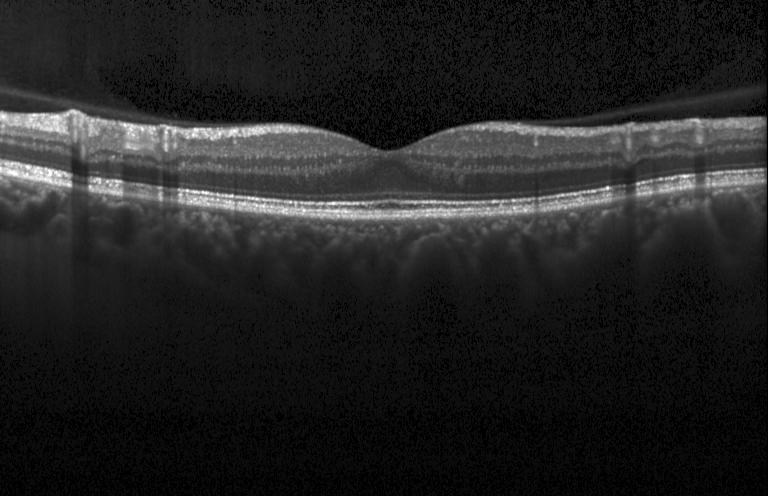
OCT scan showing no evidence of choroidal neovascularization, diabetic macular edema, or drusen.